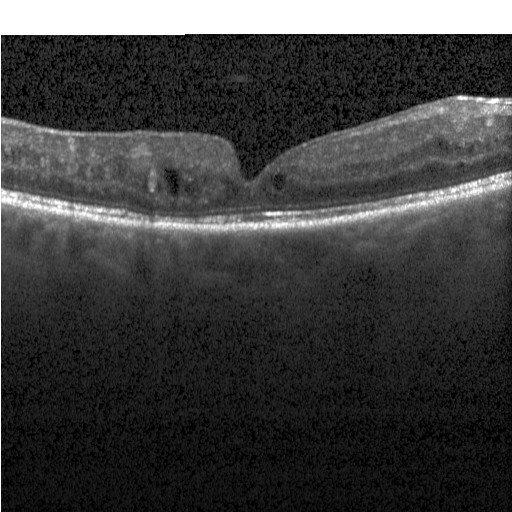
OCT line scan · Heidelberg Spectralis OCT system. OCT finding: diabetic macular edema (DME).